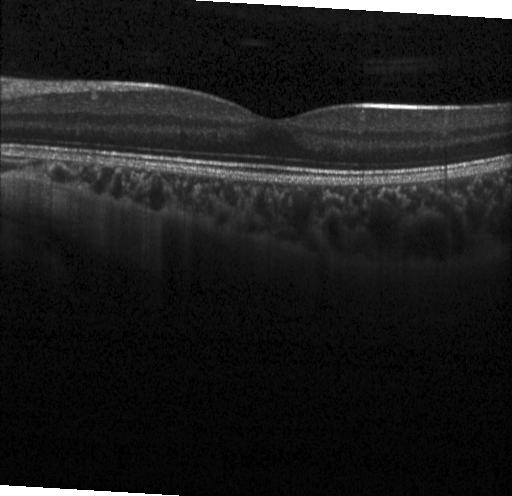 Fovea-centered · retinal OCT cross-section · spectral-domain optical coherence tomography.
Assessment: neither CNV, DME, nor drusen.